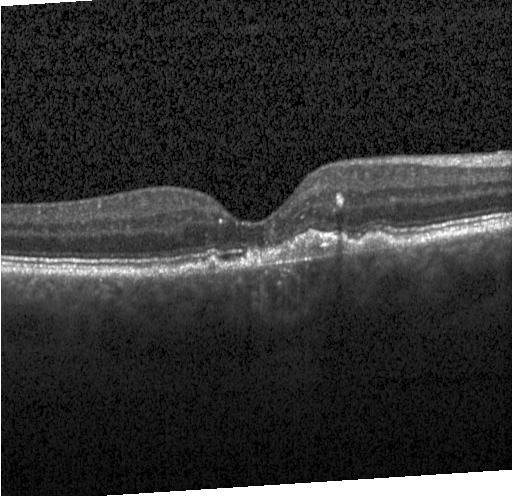

Centered on the fovea, SD-OCT, retinal OCT cross-section.
Impression: choroidal neovascularization.